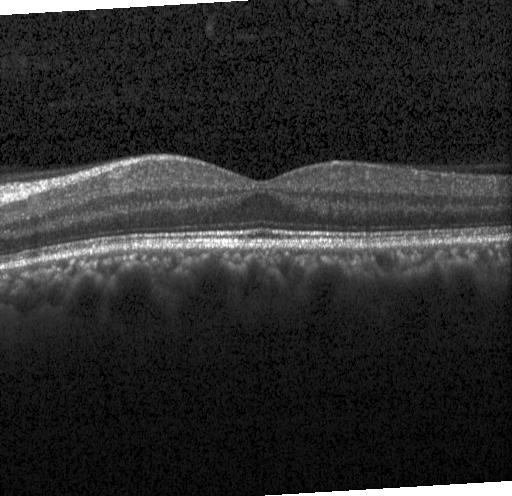 OCT B-scan. Impression: no choroidal neovascularization, diabetic macular edema, or drusen.